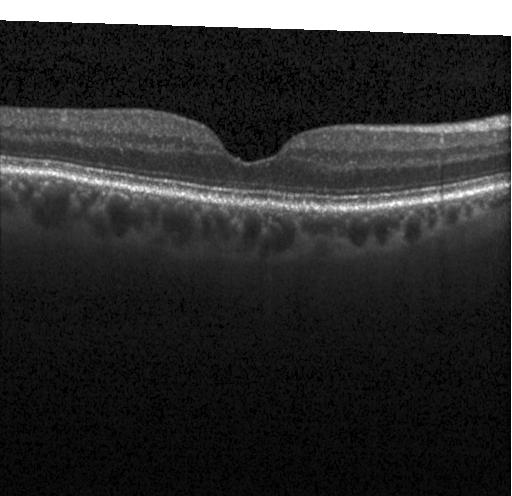
Spectral-domain OCT B-scan: no evidence of choroidal neovascularization, diabetic macular edema, or drusen.